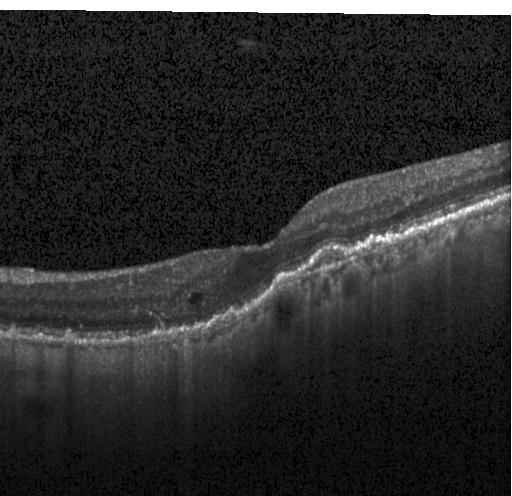

Retinal OCT cross-section. Macular scan. Finding: a choroidal neovascular membrane.